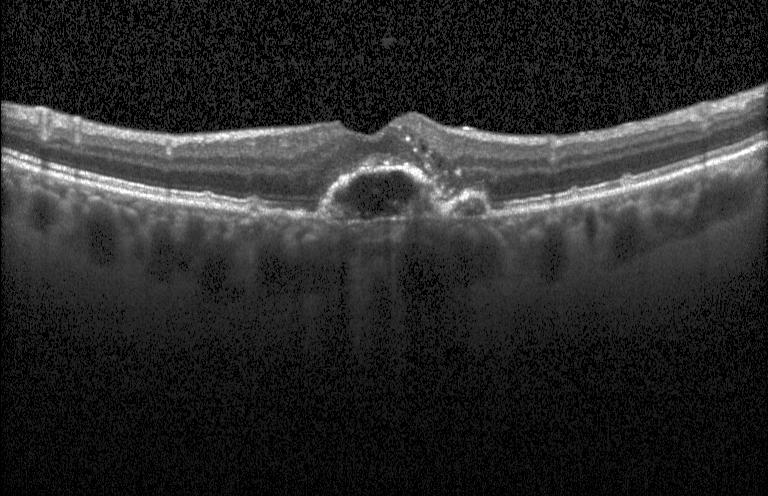
Finding: a choroidal neovascular membrane.